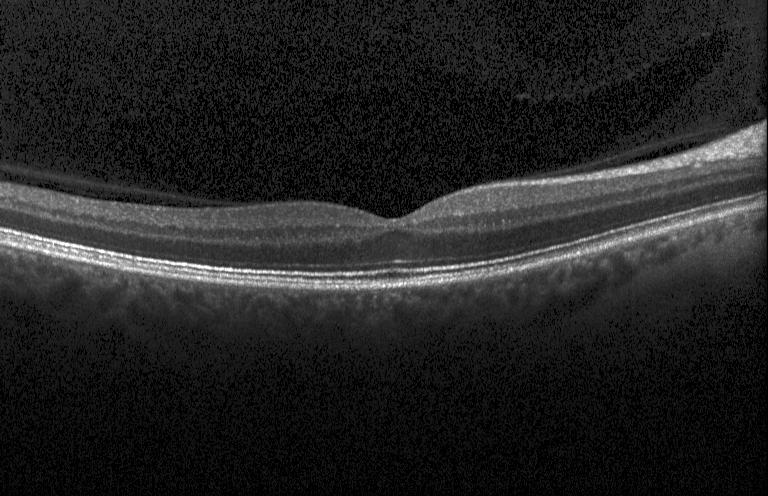 Spectral-domain OCT B-scan: no choroidal neovascularization, diabetic macular edema, or drusen.